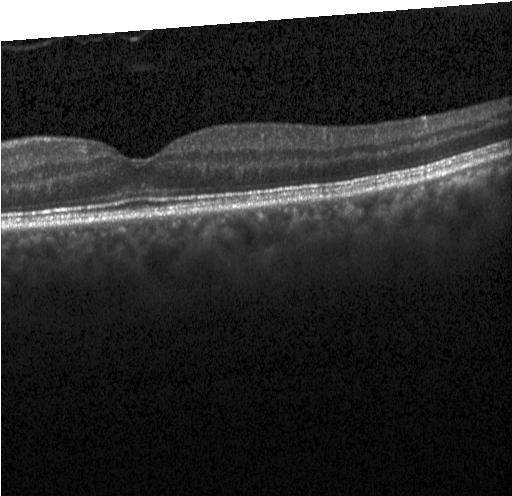 OCT finding: neither choroidal neovascularization, diabetic macular edema, nor drusen.